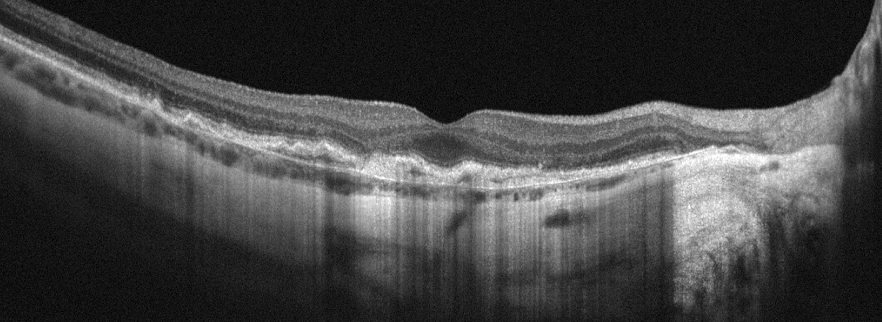
Optical coherence tomography B-scan. OD
Diagnosis: age-related macular degeneration (AMD).